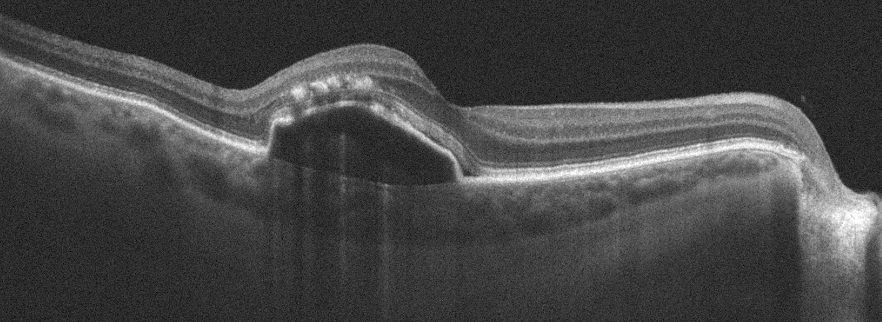
Retinal OCT B-scan
Diagnosis: age-related macular degeneration.